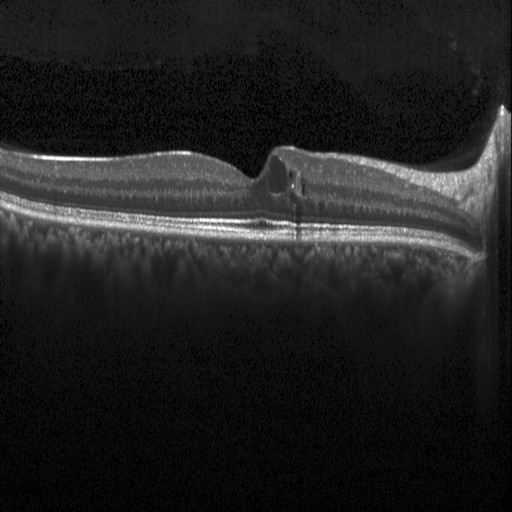 This B-scan demonstrates diabetic macular edema (DME).